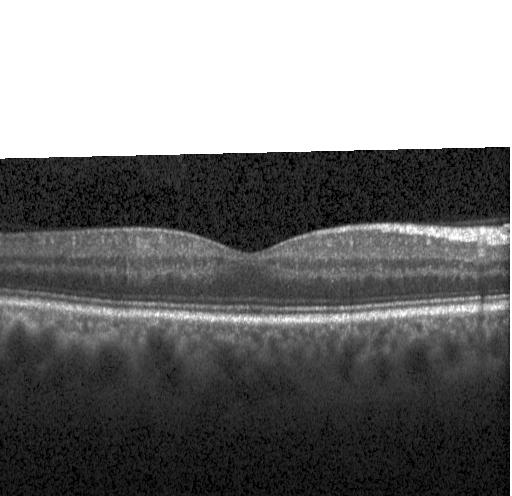

OCT B-scan
The scan shows no evidence of choroidal neovascularization, diabetic macular edema, or drusen.